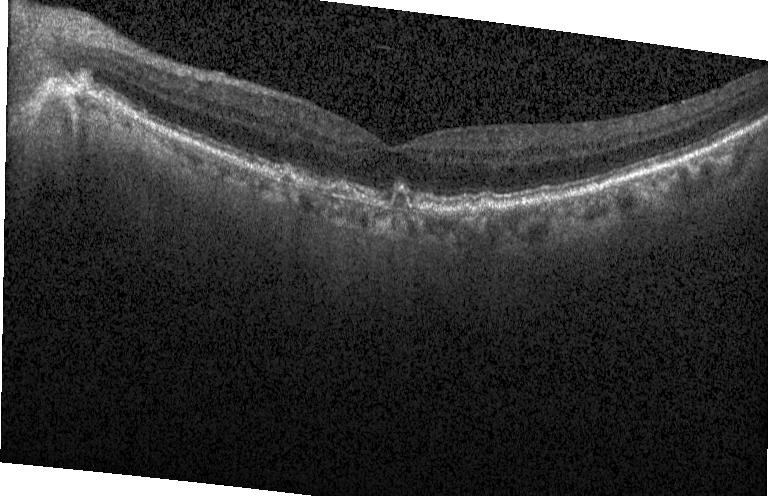
Dx: drusen.